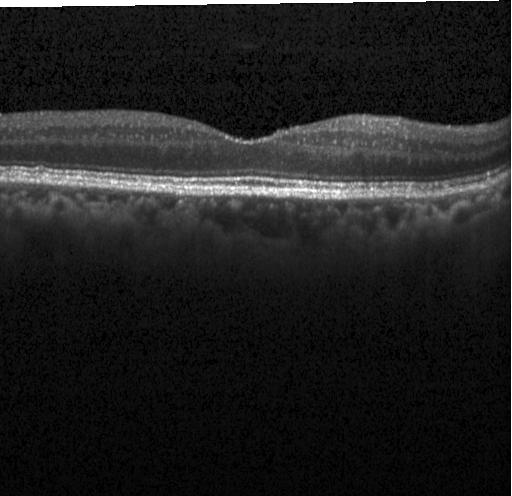 Retinal OCT B-scan. Spectral-domain OCT. Instrument: Heidelberg Spectralis. Finding: neither CNV, DME, nor drusen.